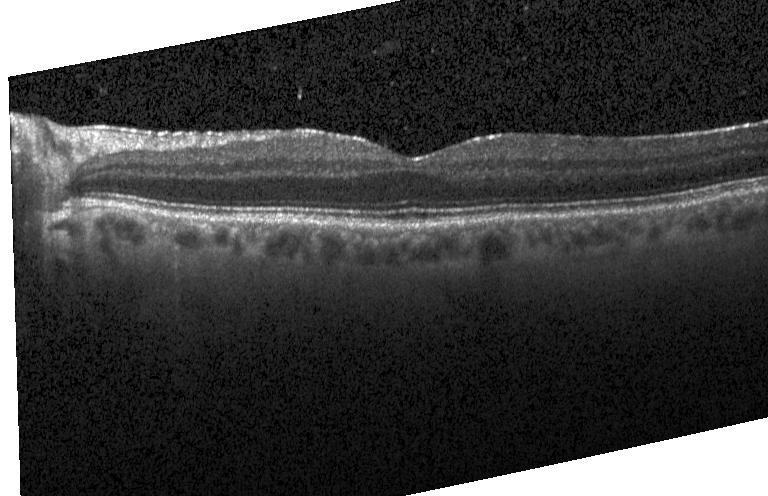 Assessment: neither choroidal neovascularization, diabetic macular edema, nor drusen.